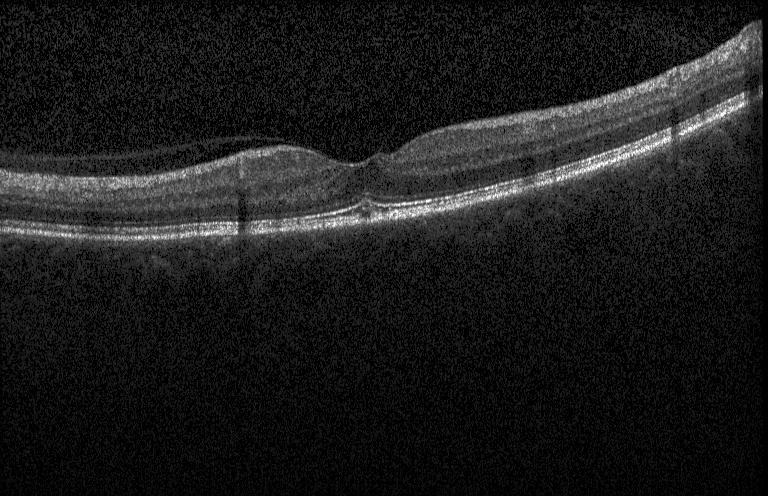
Retinal OCT cross-section
Diagnosis: no CNV, no DME, and no drusen.